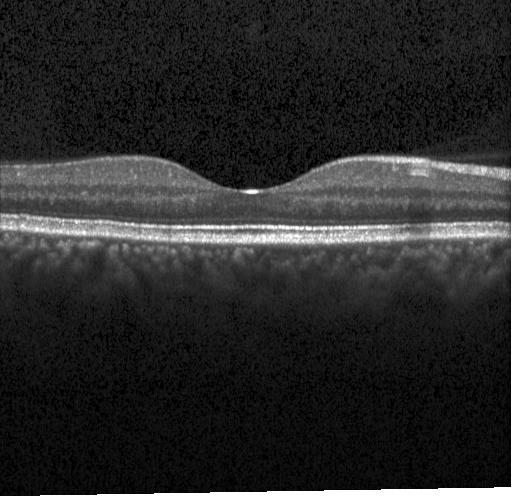

Dx: neither choroidal neovascularization, diabetic macular edema, nor drusen.